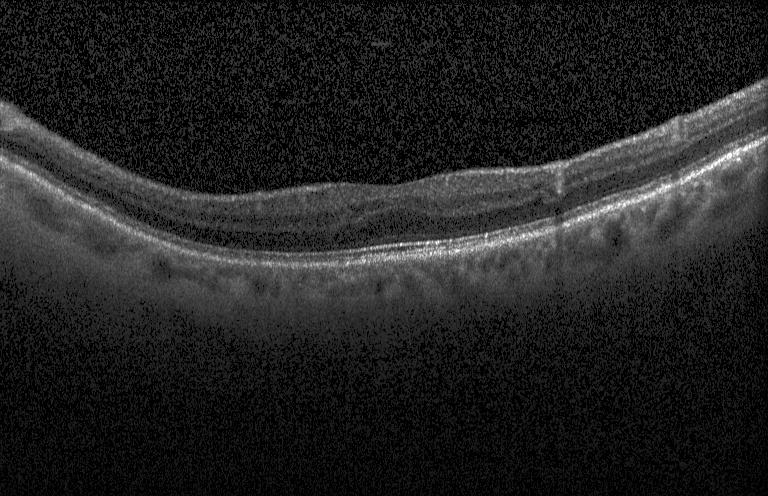 OCT line scan.
Diagnosis: neither CNV, DME, nor drusen.